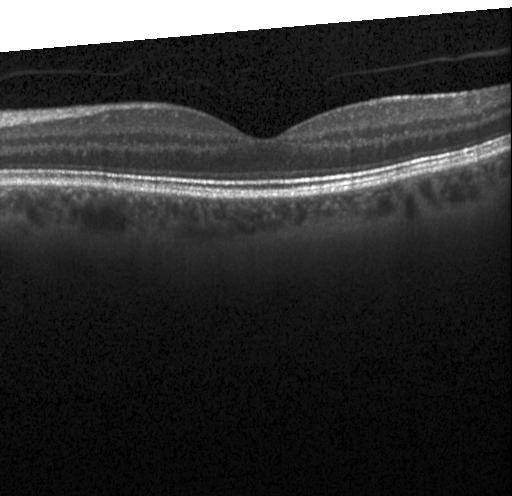

Optical coherence tomography scan. No evidence of choroidal neovascularization, diabetic macular edema, or drusen.